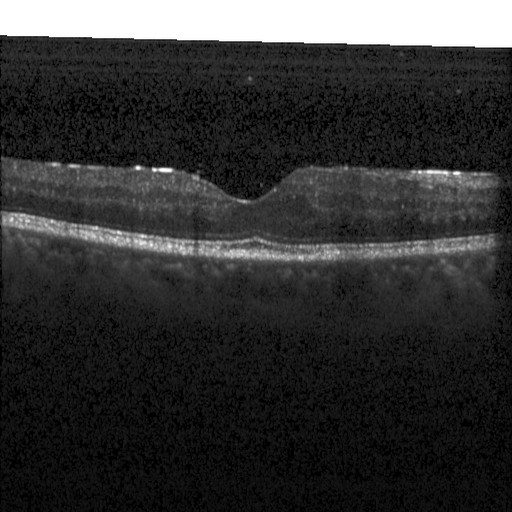

Through the macula · retinal OCT cross-section. Diagnosis: diabetic macular edema.